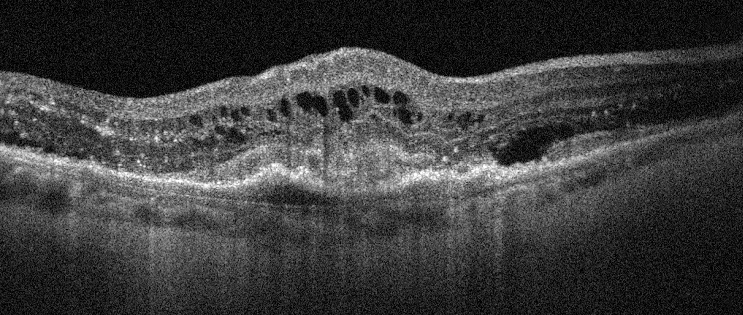
Age-related macular degeneration (AMD).